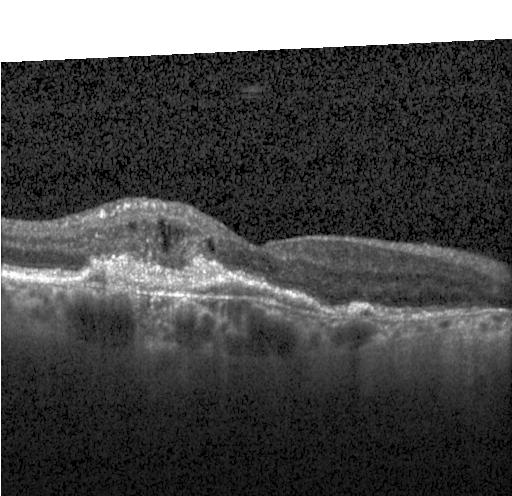 OCT B-scan showing choroidal neovascularization.